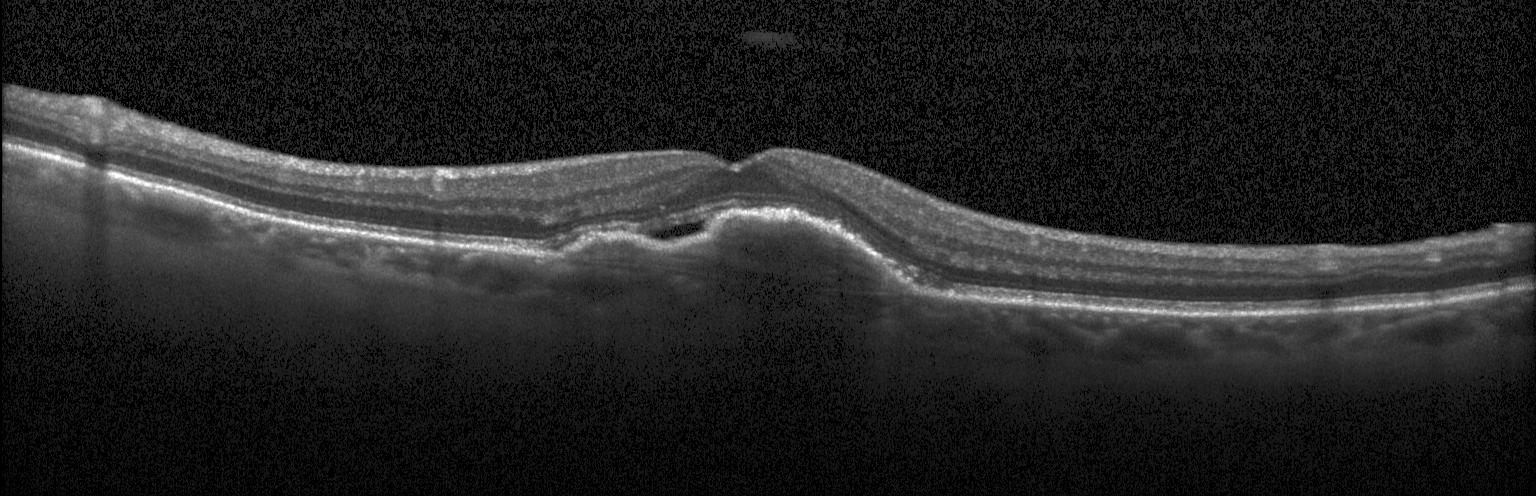 Macular OCT: a choroidal neovascular membrane.